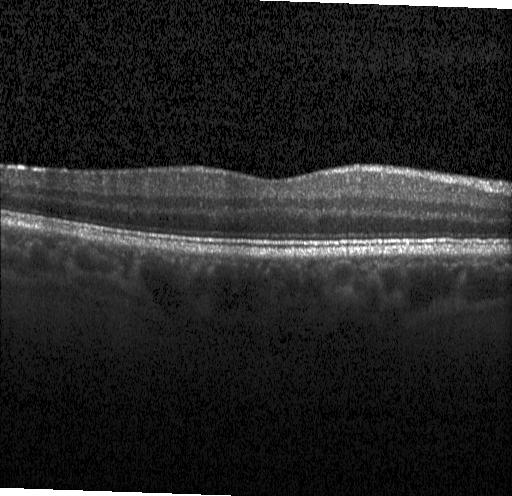

Heidelberg Spectralis · OCT B-scan.
No choroidal neovascularization, diabetic macular edema, or drusen.